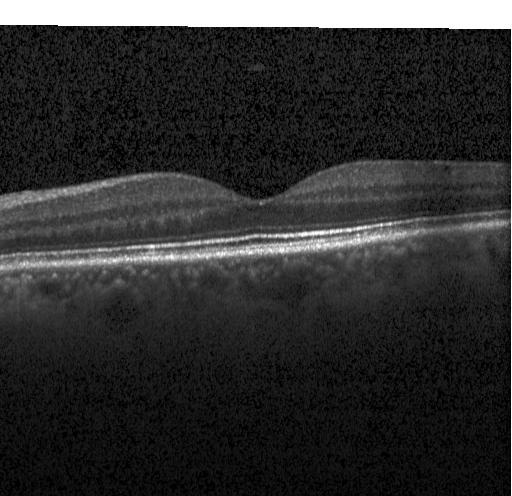

Optical coherence tomography scan — Assessment: no choroidal neovascularization, diabetic macular edema, or drusen.